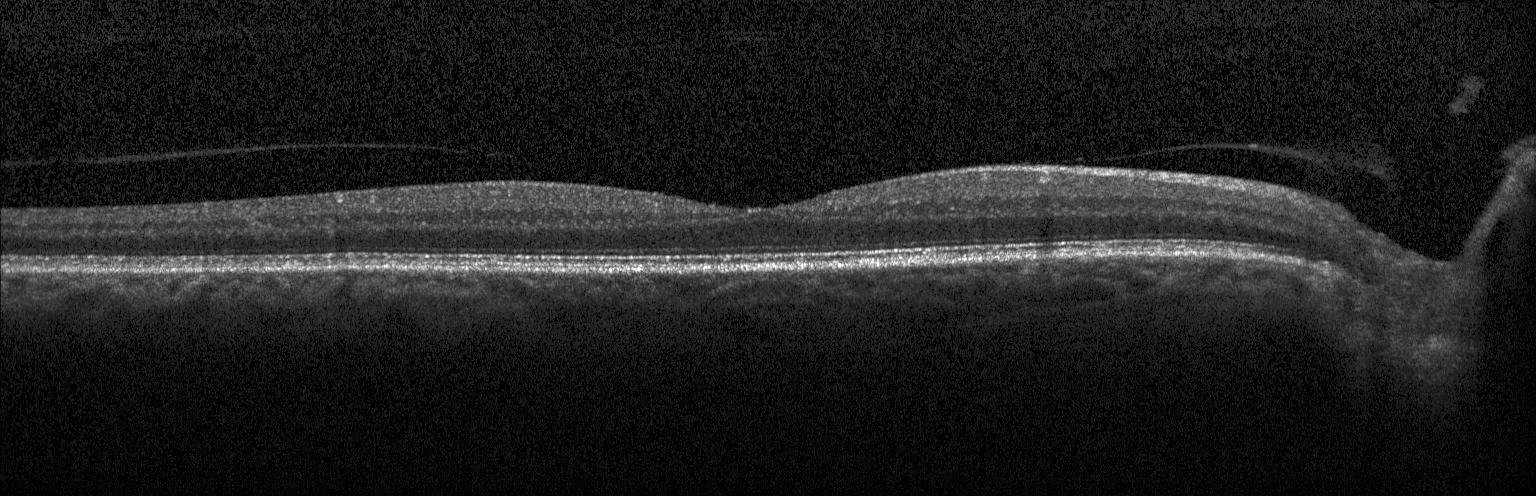
Retinal OCT cross-section; acquired on a Heidelberg Spectralis.
The scan shows neither choroidal neovascularization, diabetic macular edema, nor drusen.